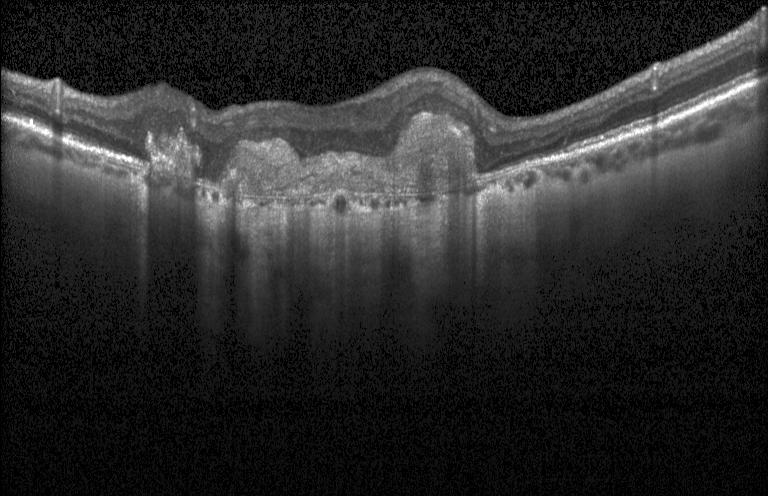 Impression: choroidal neovascularization (CNV).